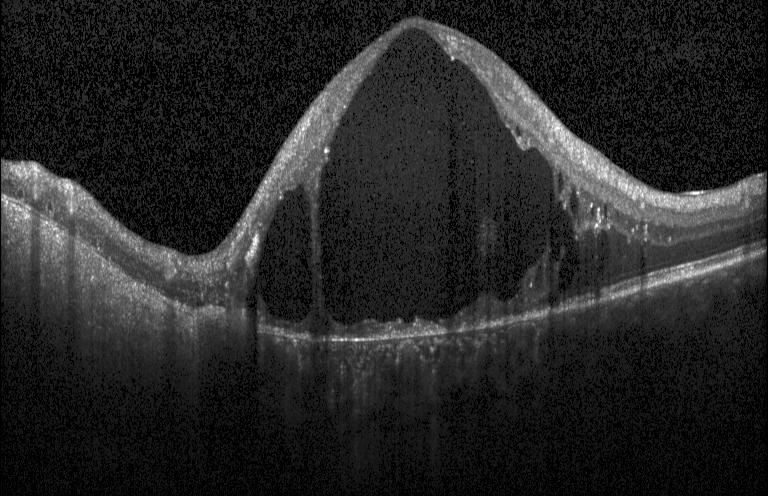

Diagnosis: diabetic macular edema (DME).